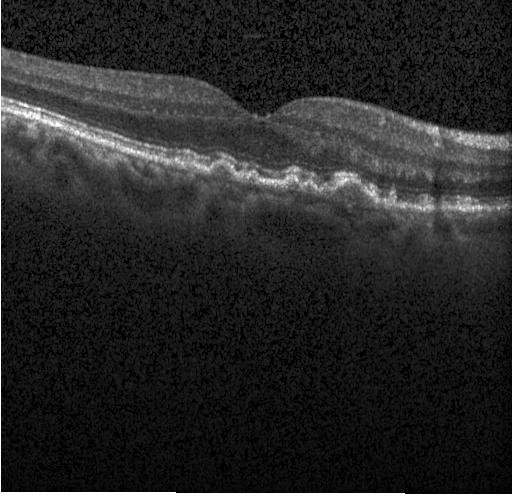 This B-scan demonstrates drusen.